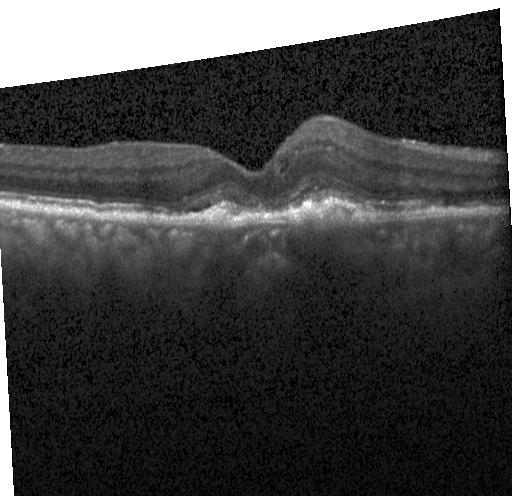 Impression: a choroidal neovascular membrane.